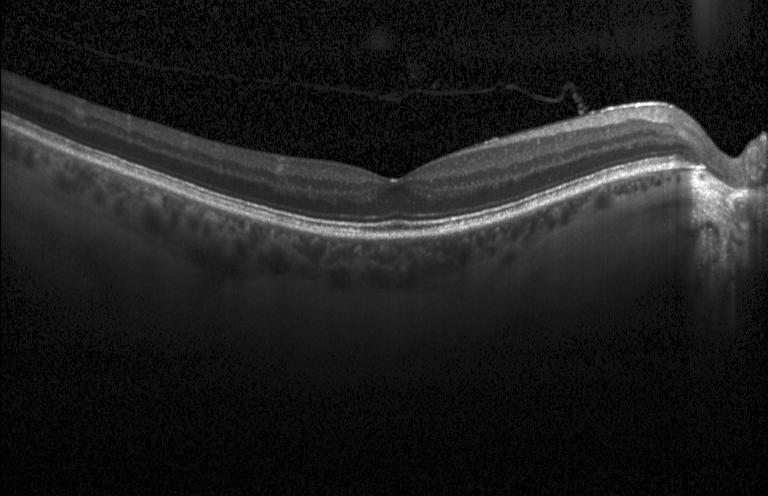 Optical coherence tomography B-scan
This B-scan demonstrates neither CNV, DME, nor drusen.